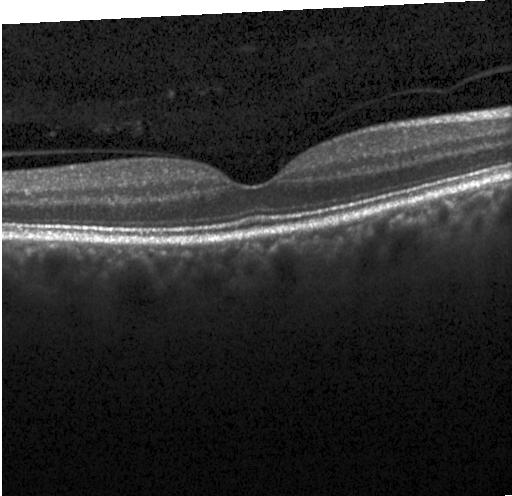

Spectral-domain OCT B-scan: no CNV, DME, or drusen.